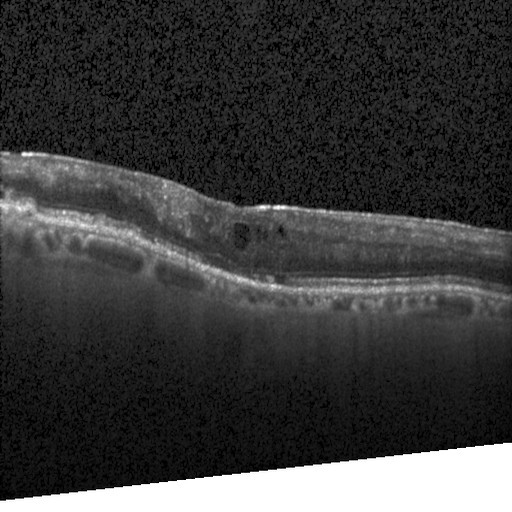

This B-scan demonstrates diabetic macular edema.